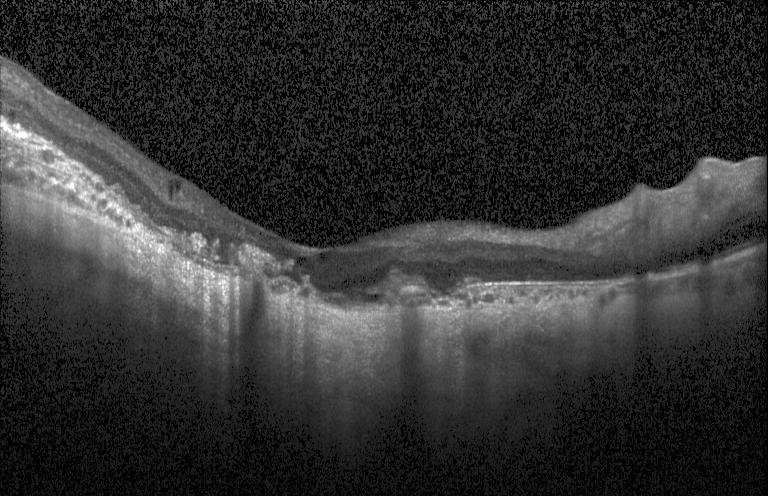
Diagnosis: choroidal neovascularization.